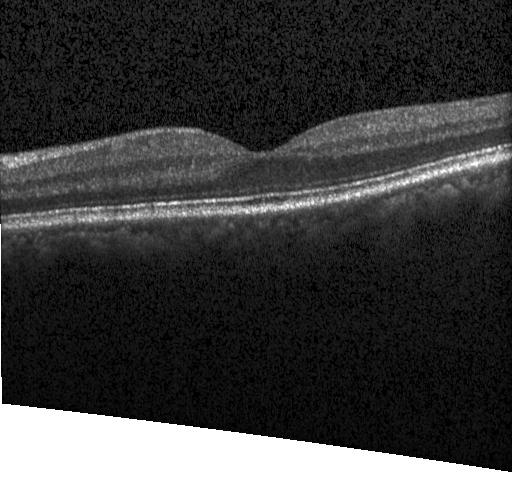

OCT finding: no choroidal neovascularization, diabetic macular edema, or drusen.